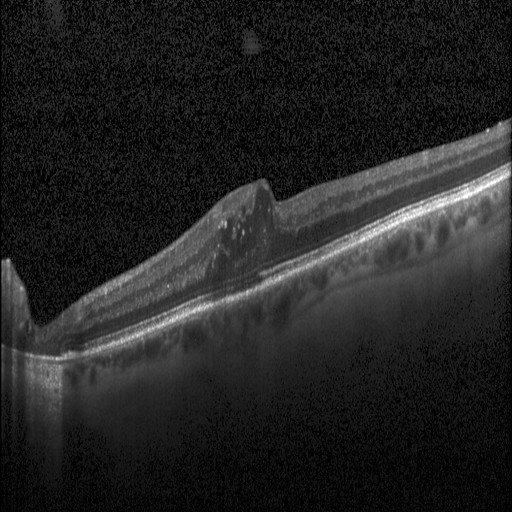

Macular OCT: DME.